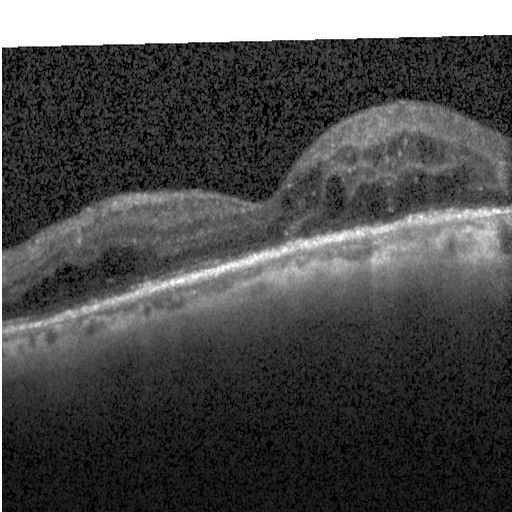

Centered on the fovea. OCT line scan. Spectral-domain optical coherence tomography. Impression: diabetic macular edema.